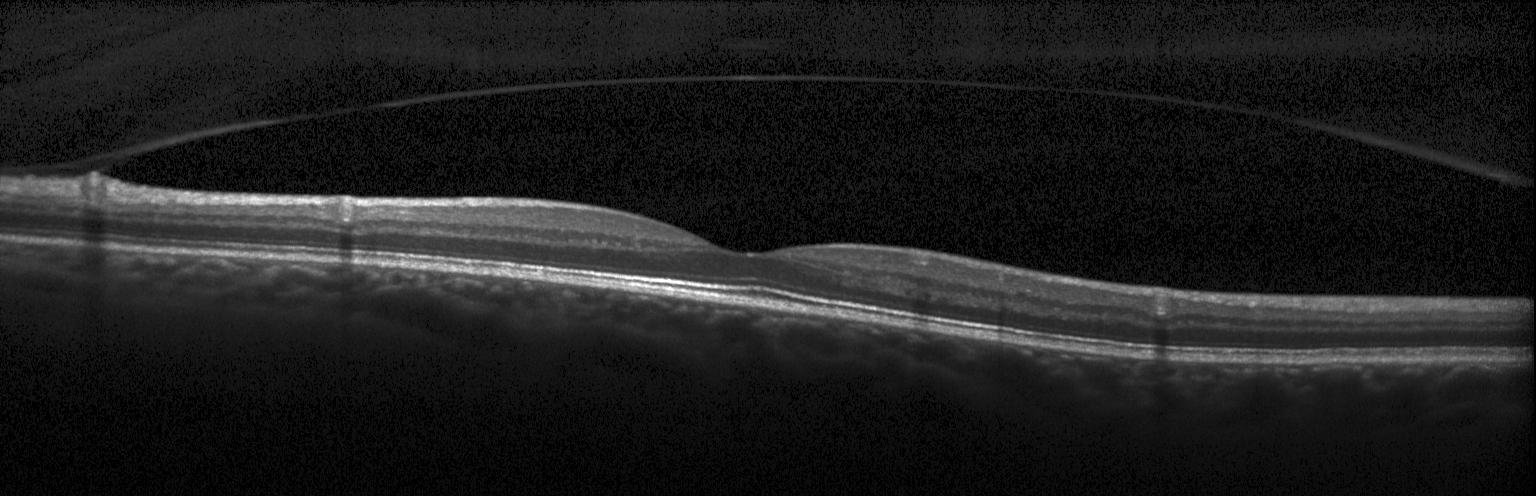

Heidelberg Spectralis OCT system · spectral-domain OCT · optical coherence tomography B-scan.
The scan shows no CNV, DME, or drusen.